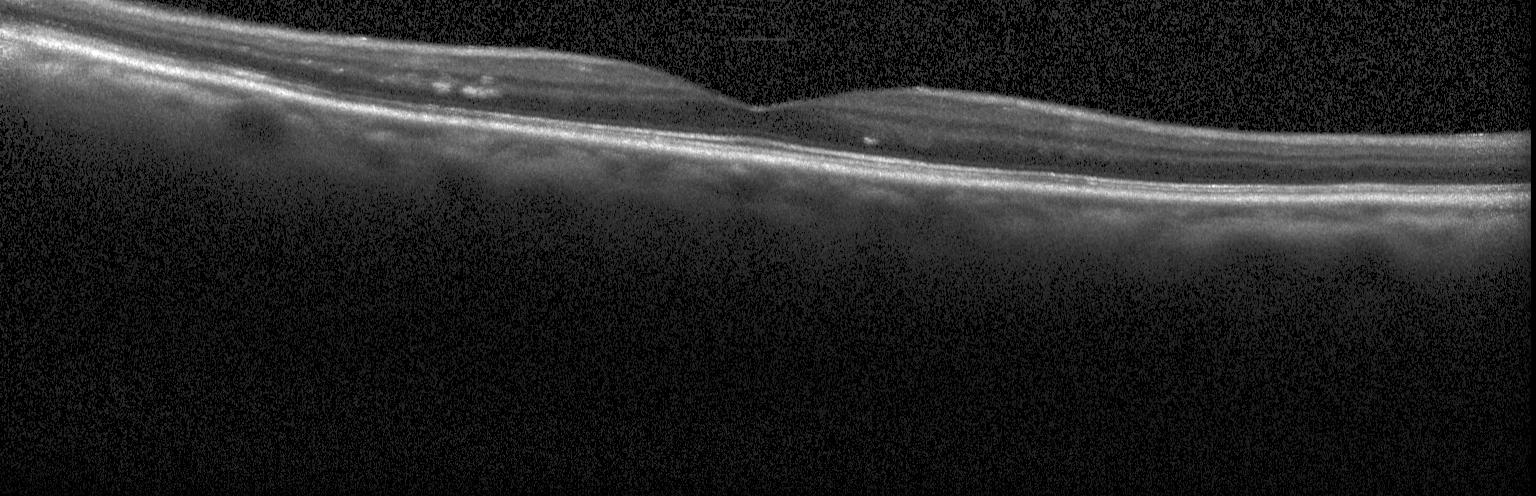
Diagnosis: no evidence of CNV, DME, or drusen.